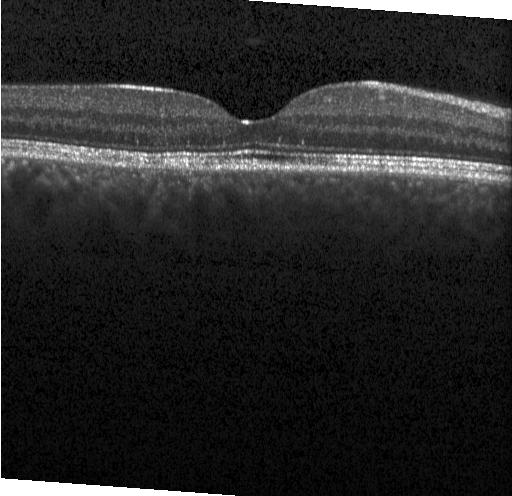

Retinal OCT cross-section. Acquired on a Heidelberg Spectralis. Spectral-domain OCT. Diagnosis: no choroidal neovascularization, diabetic macular edema, or drusen.